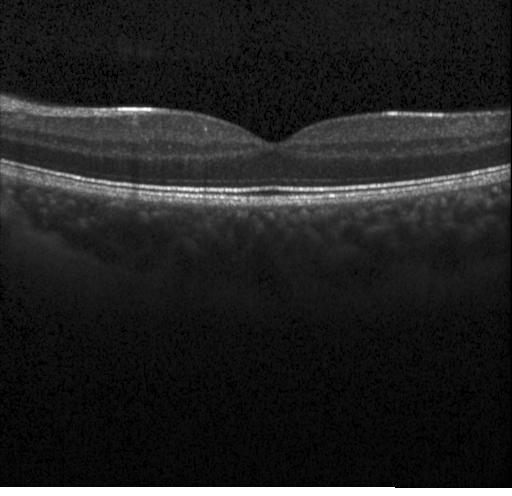

Dx: no evidence of choroidal neovascularization, diabetic macular edema, or drusen.